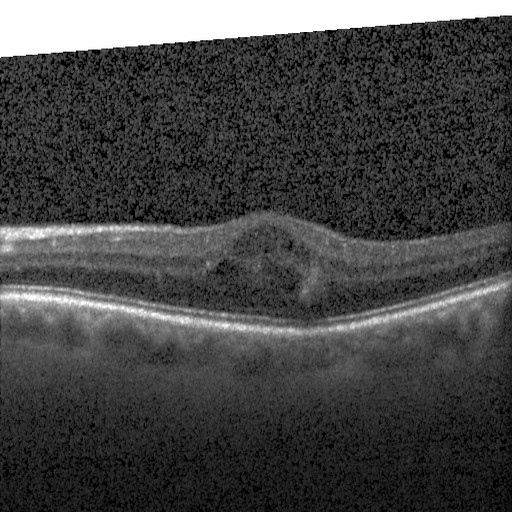 Optical coherence tomography B-scan — Diagnosis: diabetic macular edema.